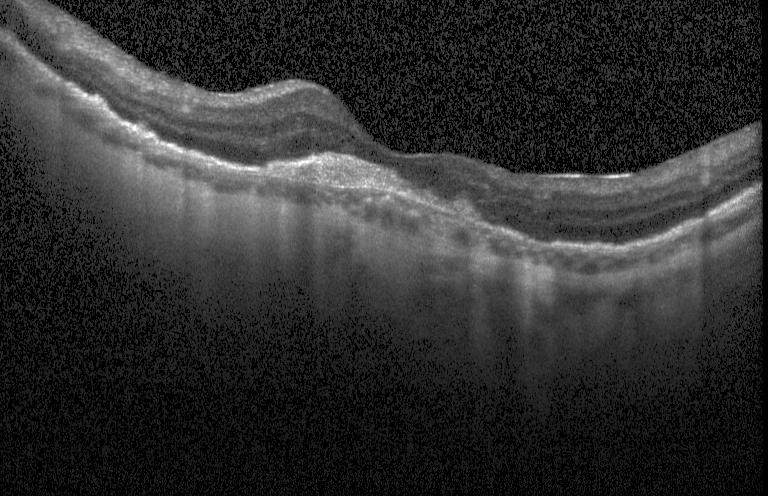
Macular OCT: a choroidal neovascular membrane.